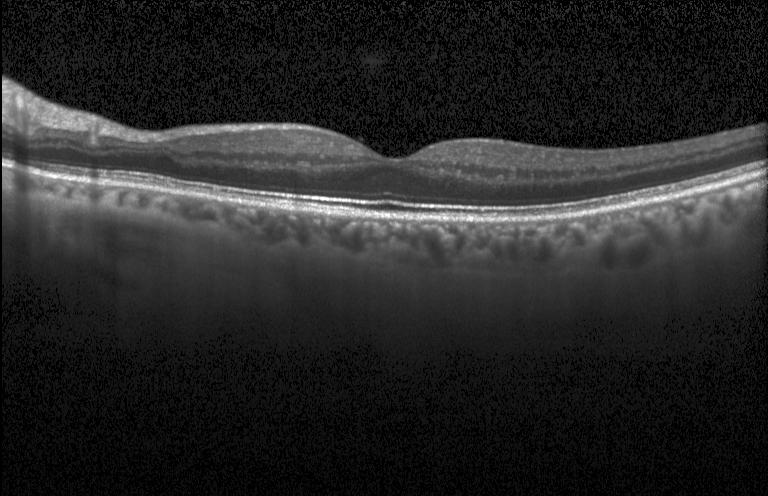

Macular OCT: no choroidal neovascularization, diabetic macular edema, or drusen.